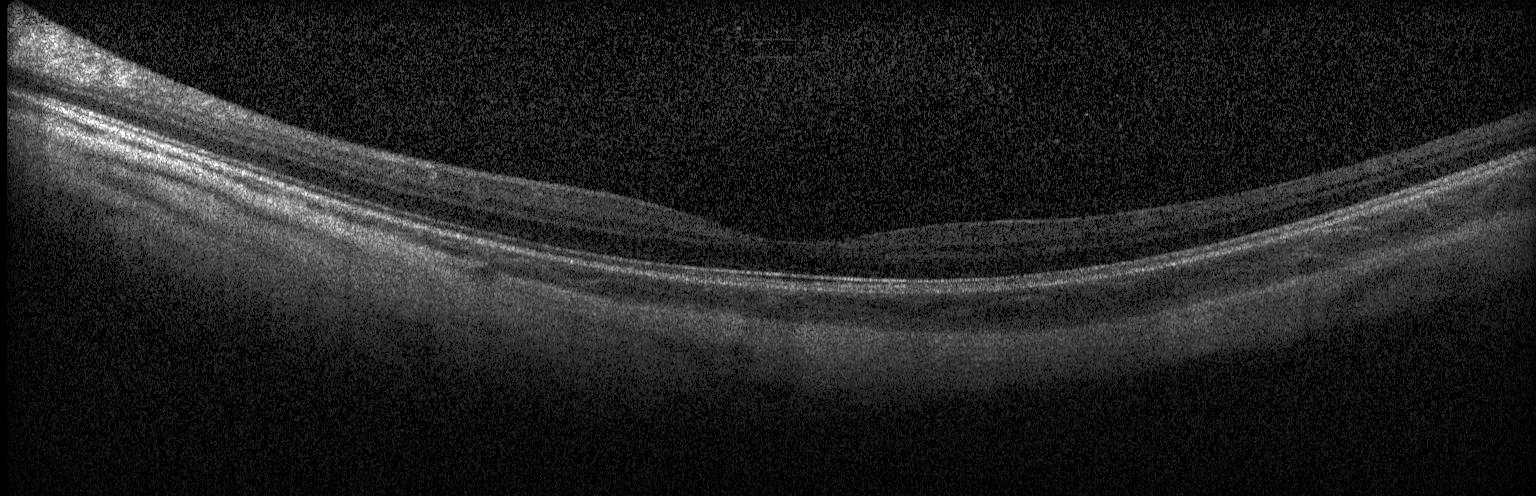 Optical coherence tomography B-scan
Dx: no evidence of choroidal neovascularization, diabetic macular edema, or drusen.